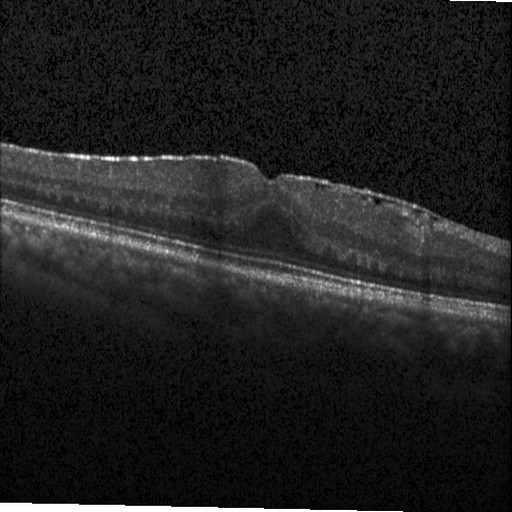

Optical coherence tomography scan
Impression: diabetic macular edema.